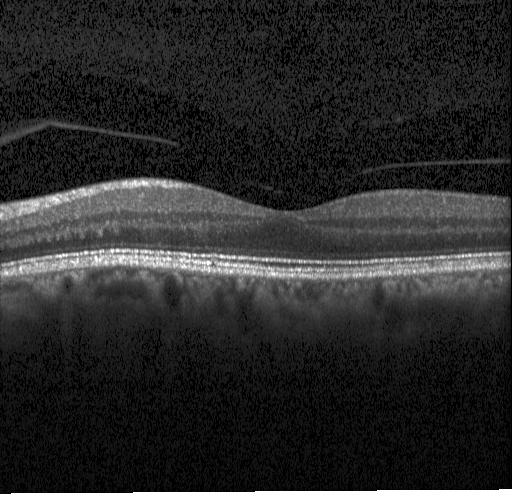
Dx: no evidence of CNV, DME, or drusen.